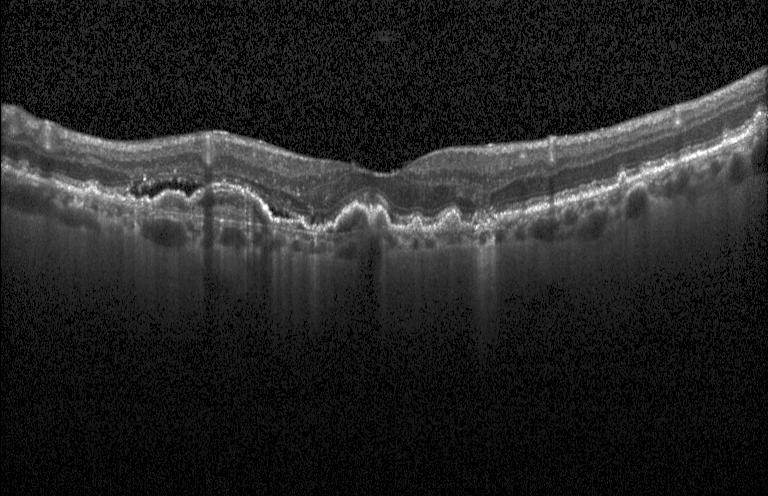
Spectral-domain OCT, OCT line scan.
Finding: a choroidal neovascular membrane.